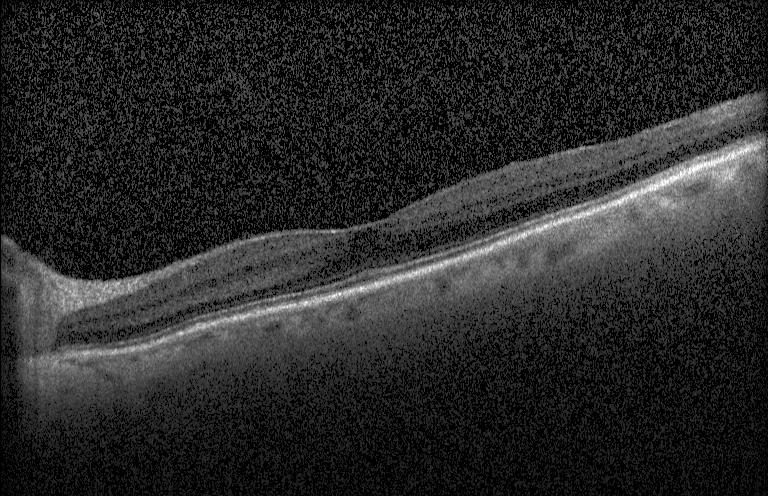

OCT scan showing no CNV, no DME, and no drusen.